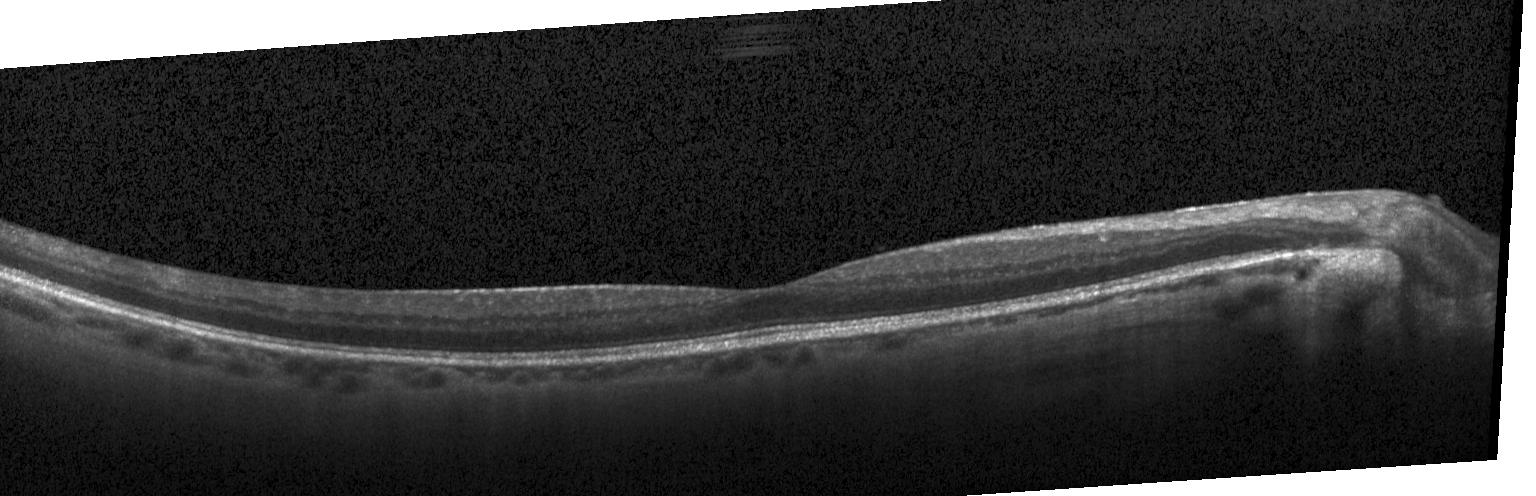
Heidelberg Spectralis, optical coherence tomography scan, macular scan.
Impression: neither CNV, DME, nor drusen.